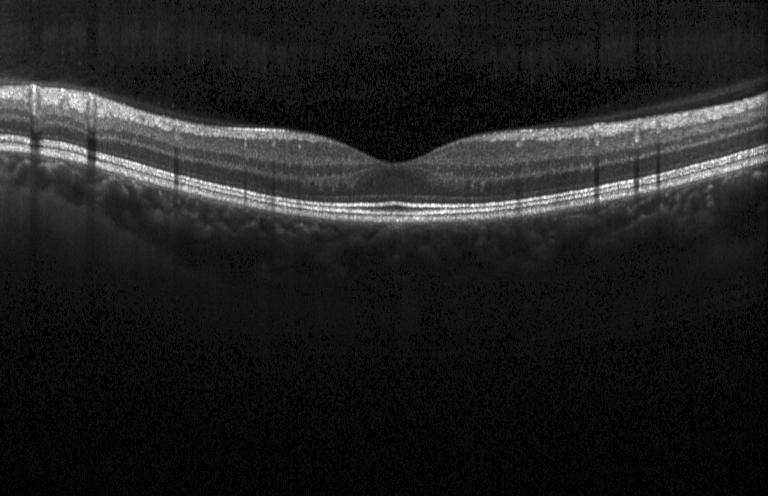

Impression: neither choroidal neovascularization, diabetic macular edema, nor drusen.